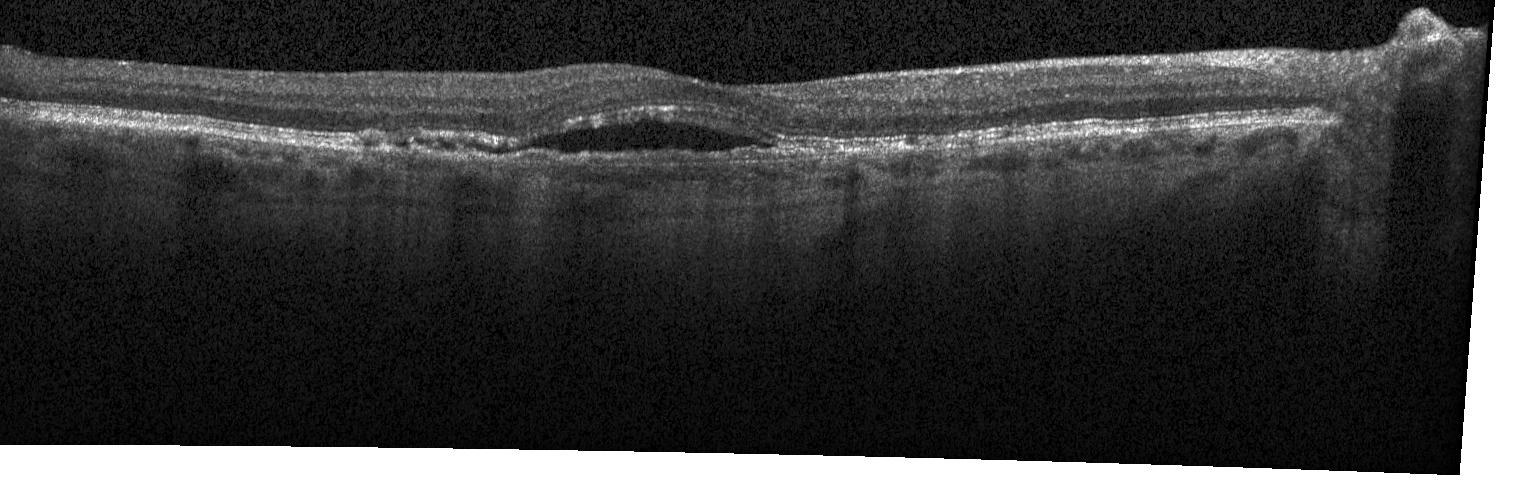

Spectral-domain OCT B-scan: a choroidal neovascular membrane.